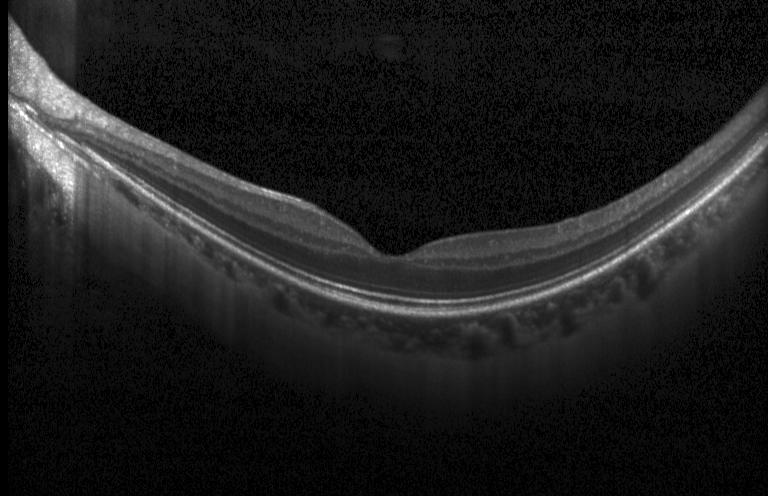 Impression: neither choroidal neovascularization, diabetic macular edema, nor drusen.